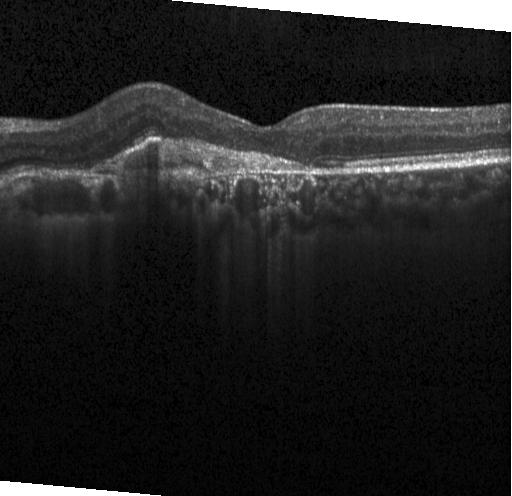

SD-OCT, retinal OCT B-scan. Impression: choroidal neovascularization.